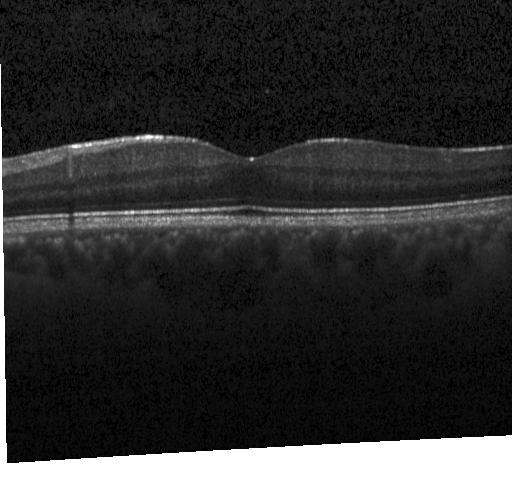
Spectral-domain optical coherence tomography. OCT line scan. Macular scan. Instrument: Heidelberg Spectralis — OCT finding: no choroidal neovascularization, diabetic macular edema, or drusen.